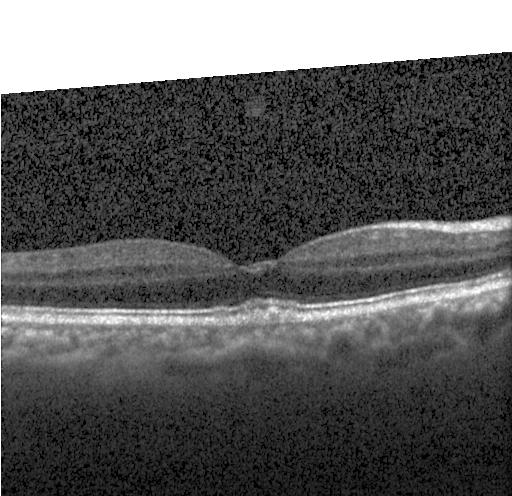

Spectral-domain OCT B-scan: drusen.